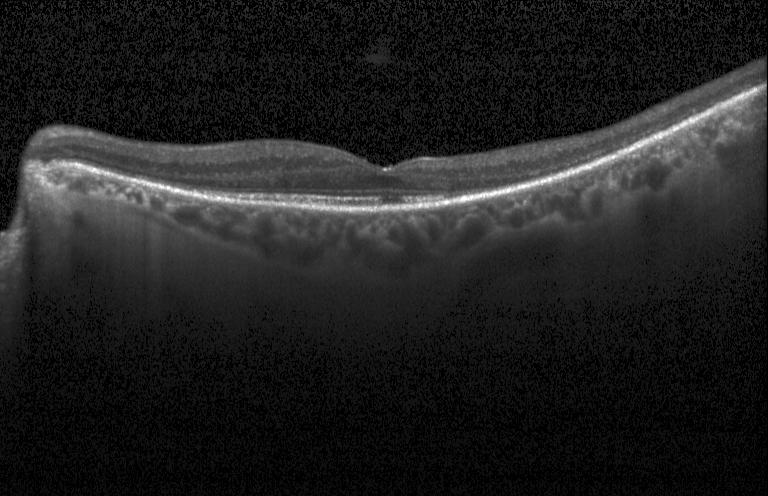 Spectral-domain OCT; Heidelberg Spectralis OCT system; optical coherence tomography B-scan; horizontal scan through the fovea
Finding: no CNV, DME, or drusen.